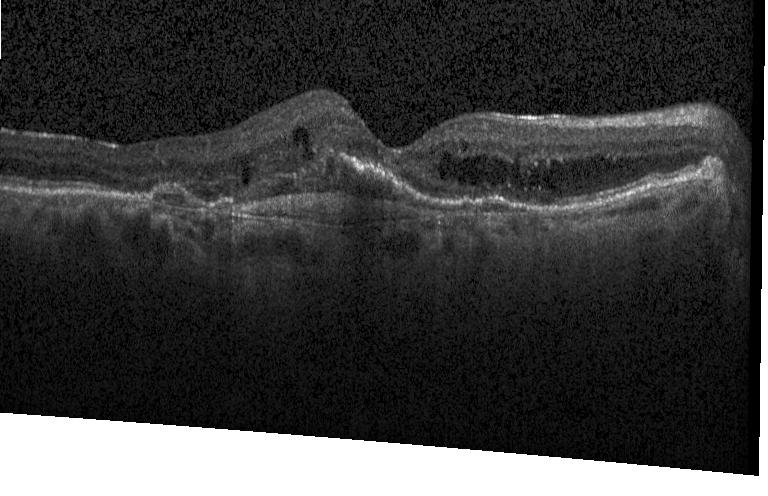

OCT B-scan
Impression: a choroidal neovascular membrane.